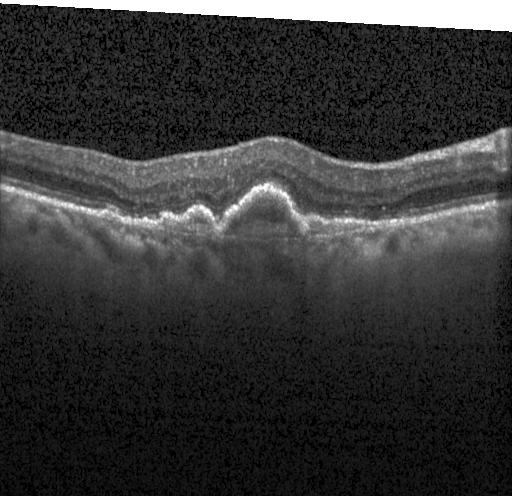

OCT line scan, spectral-domain OCT — Diagnosis: a choroidal neovascular membrane.